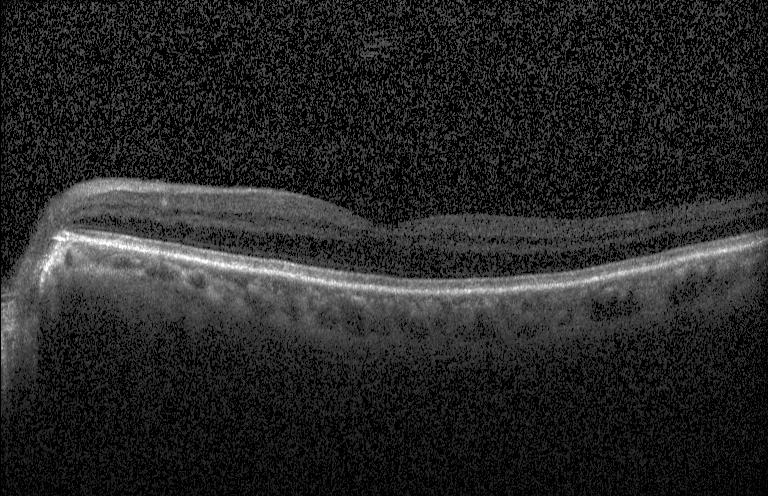 Optical coherence tomography scan. Acquired on a Heidelberg Spectralis — Impression: neither CNV, DME, nor drusen.